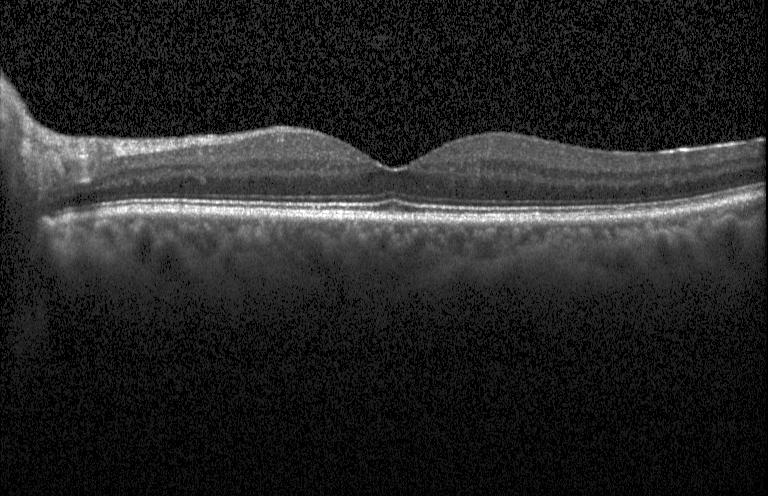

Impression: no evidence of choroidal neovascularization, diabetic macular edema, or drusen.